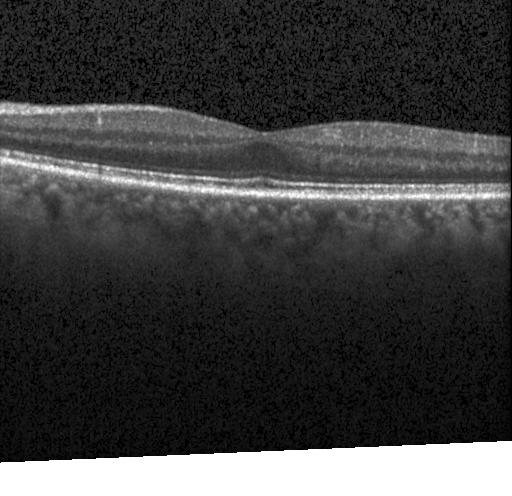 Diagnosis: neither choroidal neovascularization, diabetic macular edema, nor drusen.